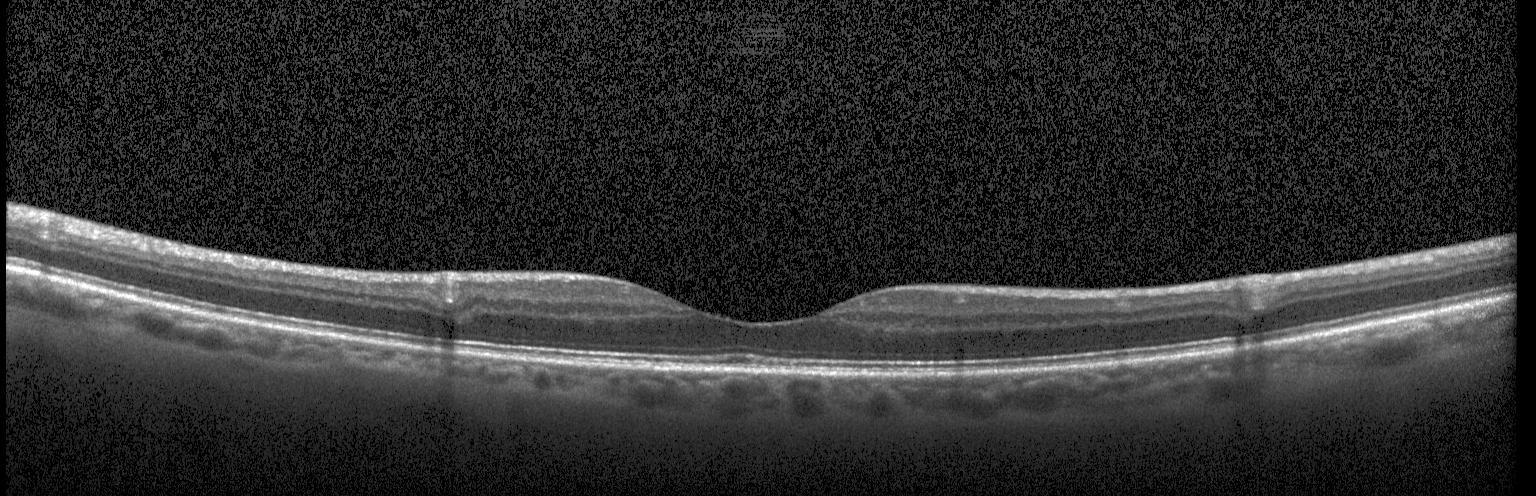

OCT B-scan.
This B-scan demonstrates no choroidal neovascularization, diabetic macular edema, or drusen.